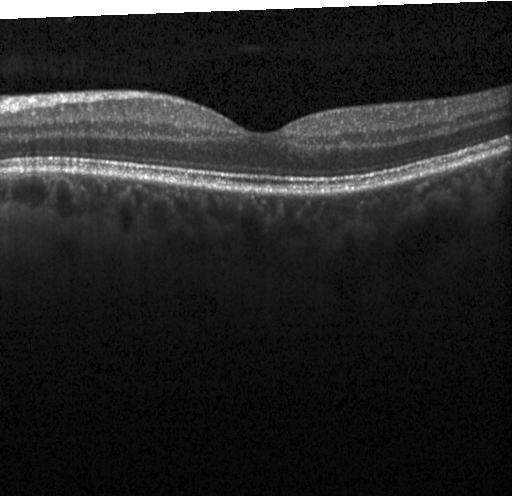 OCT B-scan, spectral-domain optical coherence tomography. Finding: no CNV, DME, or drusen.